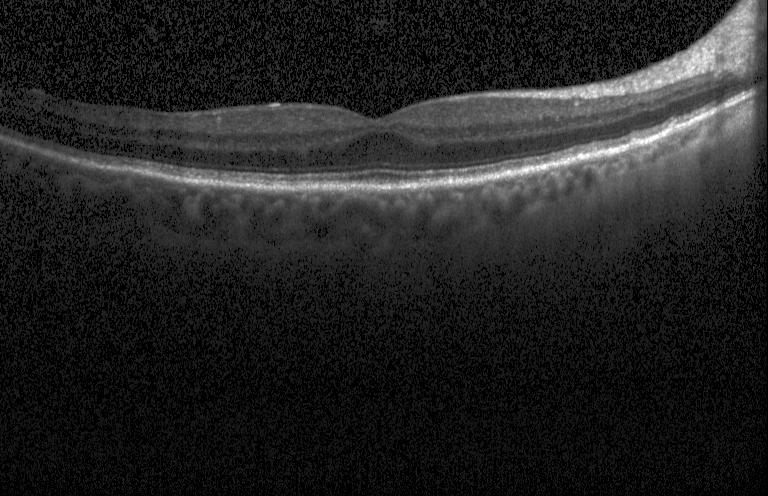

Dx: neither choroidal neovascularization, diabetic macular edema, nor drusen.